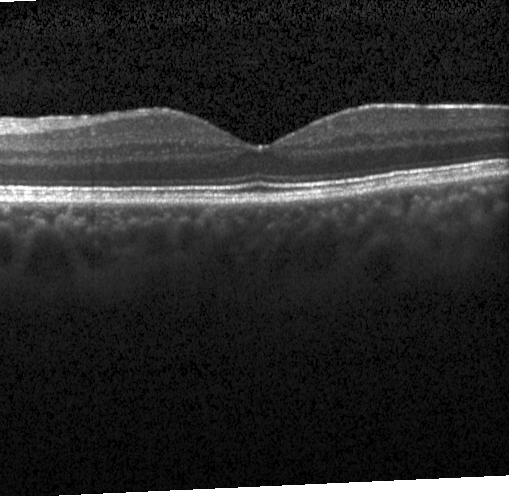

Heidelberg Spectralis. OCT line scan.
Assessment: neither choroidal neovascularization, diabetic macular edema, nor drusen.